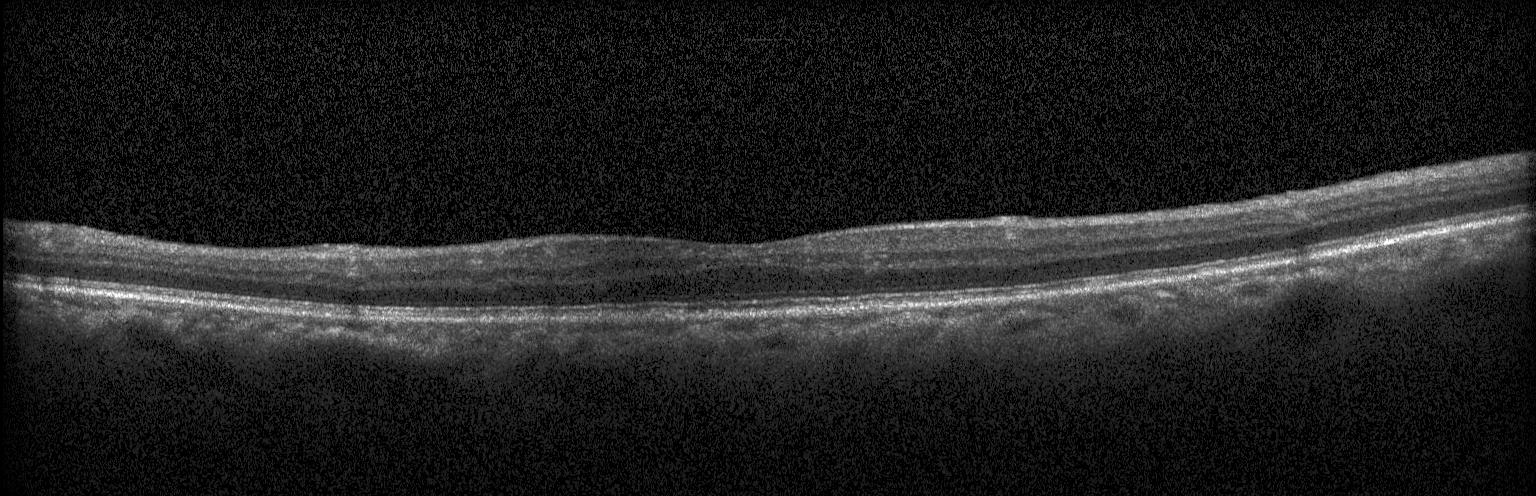

Retinal OCT cross-section; SD-OCT; instrument: Heidelberg Spectralis; macular scan
Dx: no evidence of CNV, DME, or drusen.